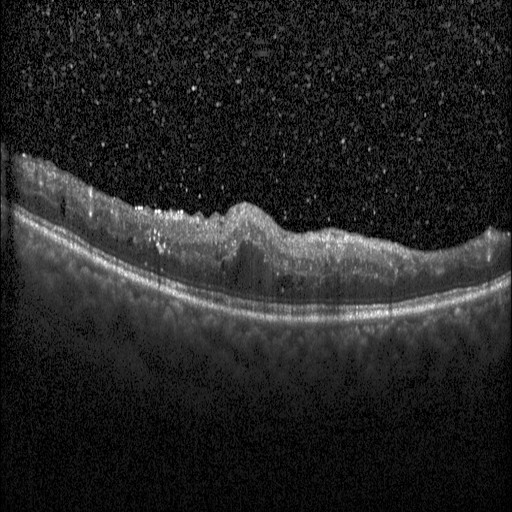 OCT B-scan showing DME.